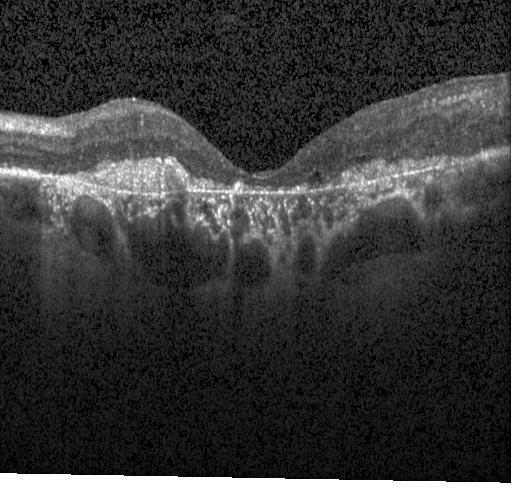

Acquired on a Heidelberg Spectralis, retinal OCT cross-section
Impression: a choroidal neovascular membrane.